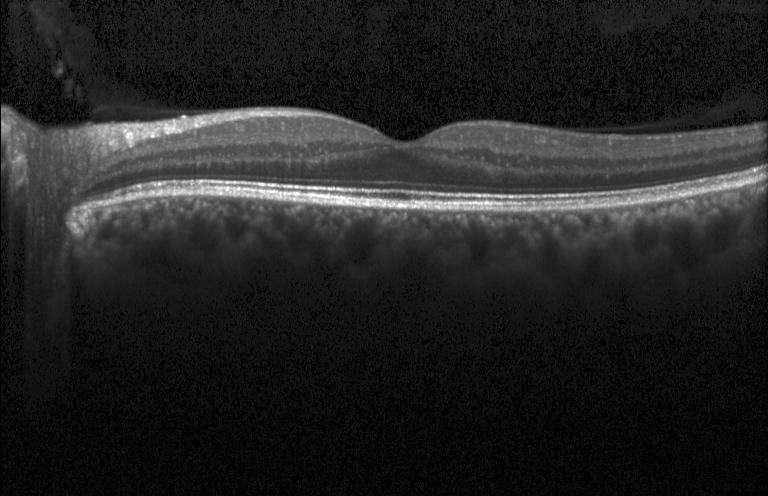 Macular OCT demonstrating neither CNV, DME, nor drusen.